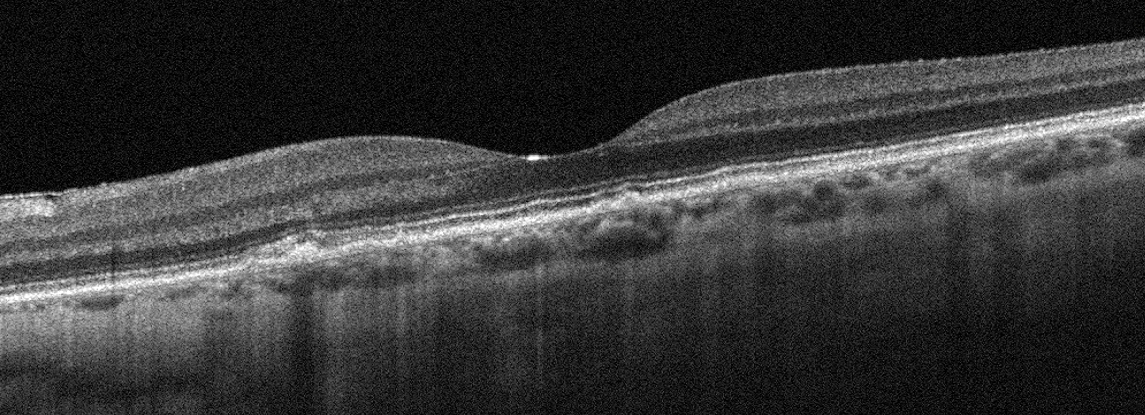

Optical coherence tomography B-scan.
Macular OCT: age-related macular degeneration (AMD).